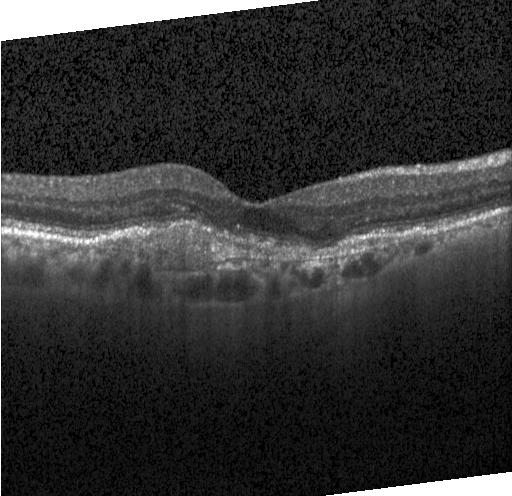

Acquired on a Heidelberg Spectralis · spectral-domain OCT · optical coherence tomography B-scan · fovea-centered. Macular OCT: choroidal neovascularization (CNV).